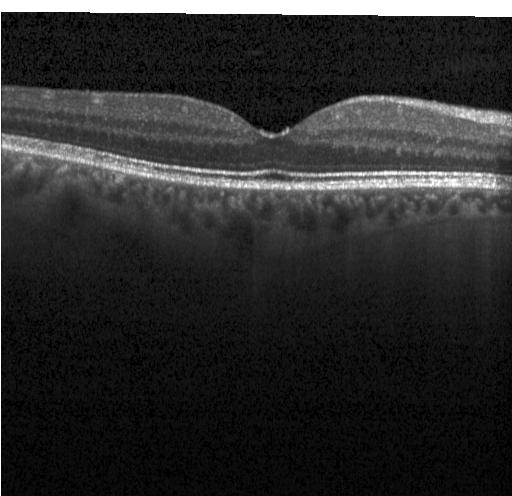 This B-scan demonstrates no choroidal neovascularization, diabetic macular edema, or drusen.